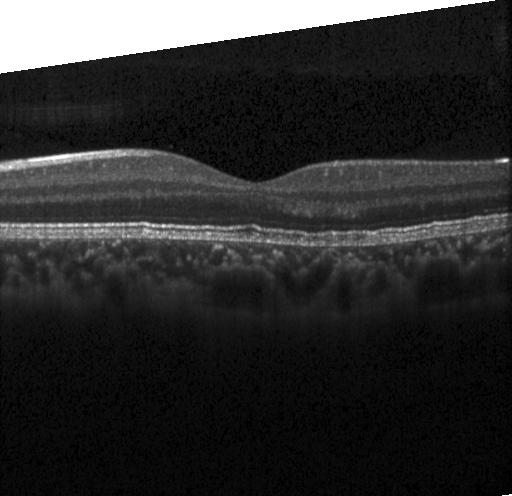

Assessment: no choroidal neovascularization, no diabetic macular edema, and no drusen.